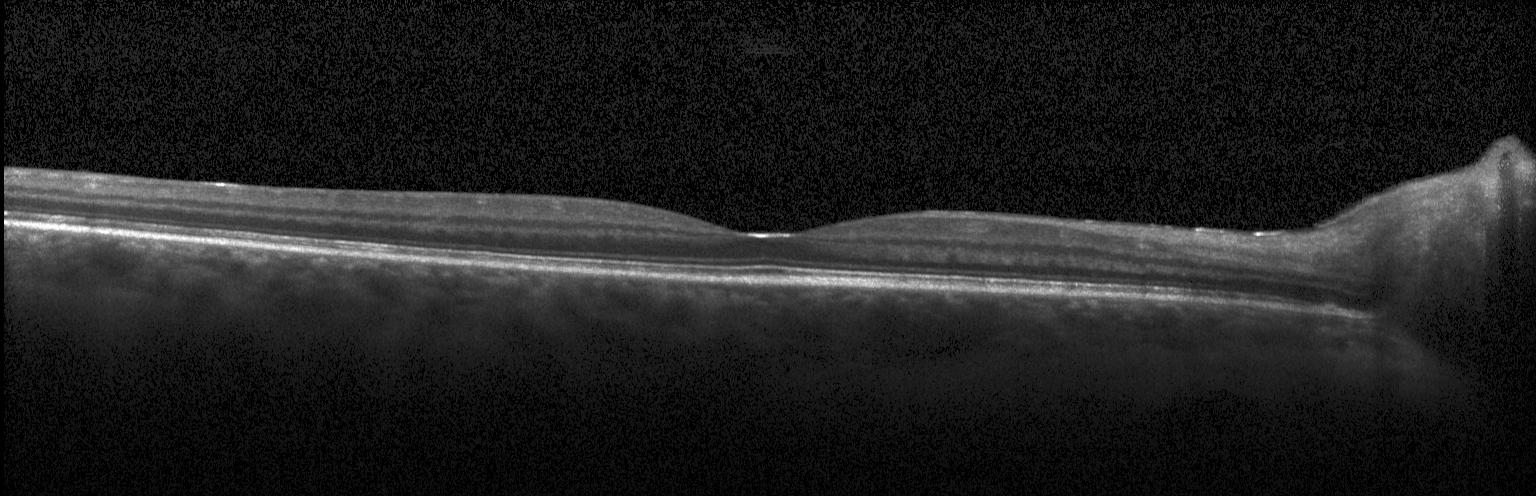 Heidelberg Spectralis · horizontal scan through the fovea · retinal OCT cross-section · spectral-domain OCT. Diagnosis: no choroidal neovascularization, diabetic macular edema, or drusen.